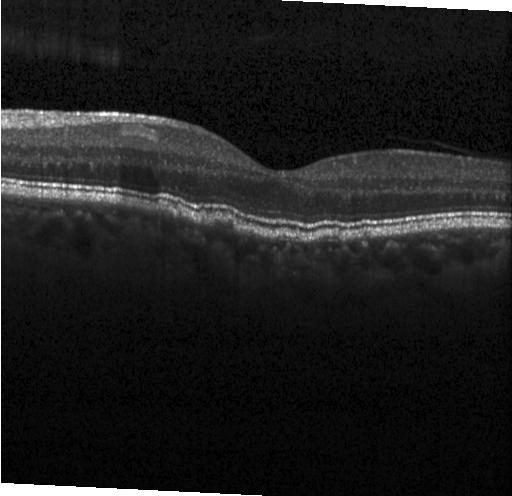 Heidelberg Spectralis, spectral-domain optical coherence tomography, optical coherence tomography scan, fovea-centered.
The scan shows multiple drusen.